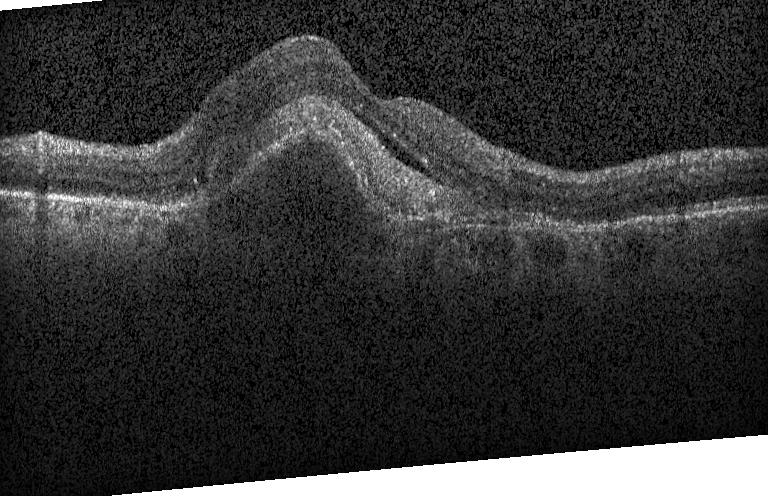 Retinal OCT B-scan · fovea-centered · spectral-domain optical coherence tomography · acquired on a Heidelberg Spectralis.
Finding: choroidal neovascularization (CNV).